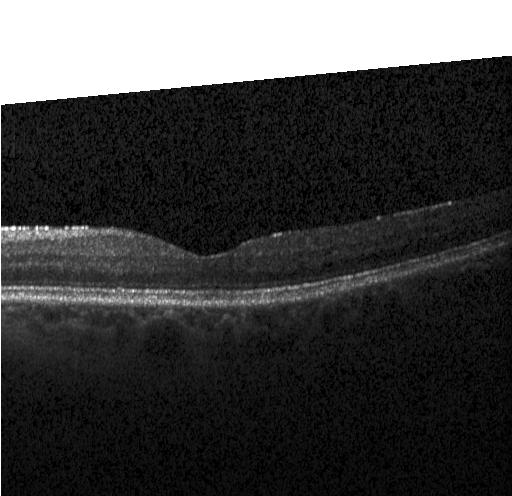 Optical coherence tomography scan. Instrument: Heidelberg Spectralis. Horizontal scan through the fovea. SD-OCT — Diagnosis: no evidence of choroidal neovascularization, diabetic macular edema, or drusen.